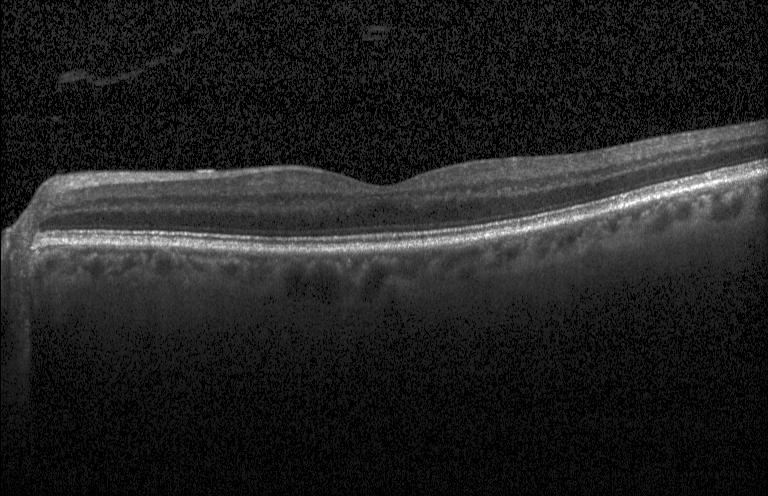
OCT finding: neither choroidal neovascularization, diabetic macular edema, nor drusen.